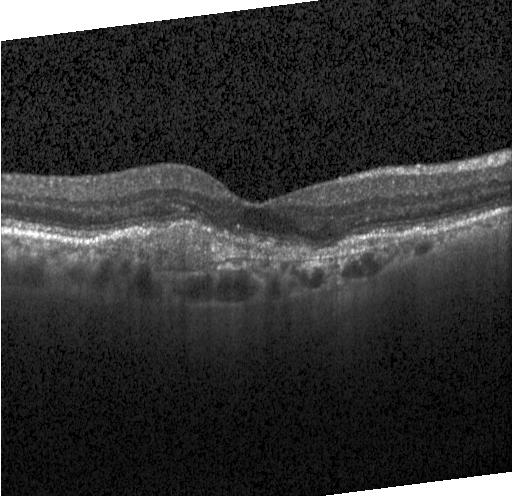 Horizontal scan through the fovea · retinal OCT B-scan · acquired on a Heidelberg Spectralis. Finding: choroidal neovascularization (CNV).